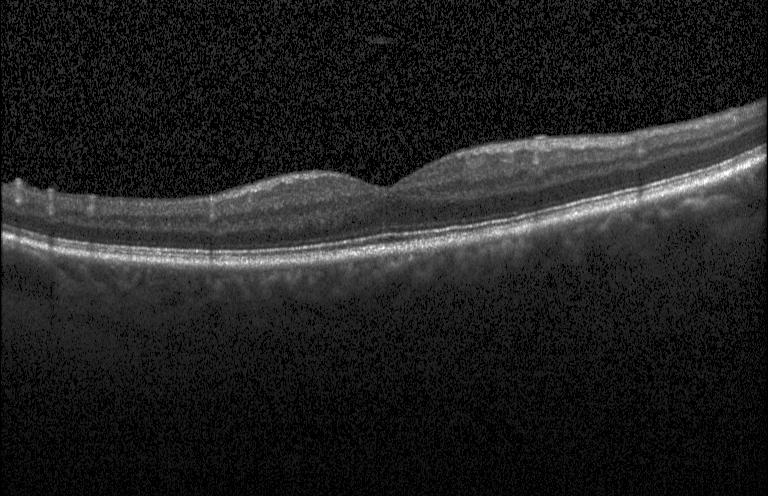 Instrument: Heidelberg Spectralis. SD-OCT. Fovea-centered. Retinal OCT cross-section — The scan shows neither choroidal neovascularization, diabetic macular edema, nor drusen.